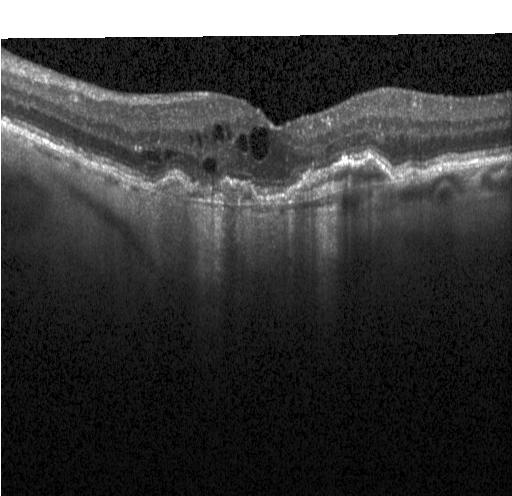
Macular OCT demonstrating choroidal neovascularization.